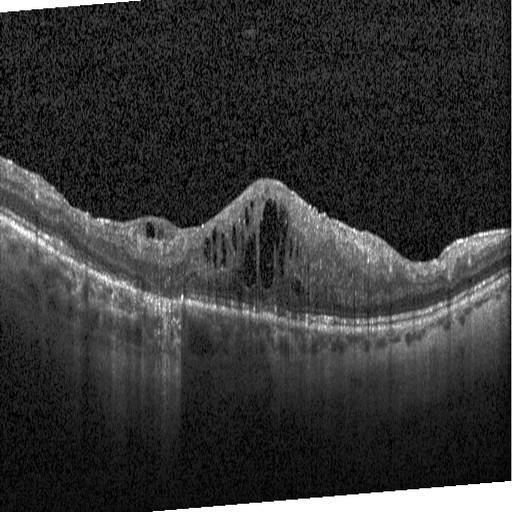
Macular scan · instrument: Heidelberg Spectralis · optical coherence tomography B-scan
Assessment: diabetic macular edema (DME).